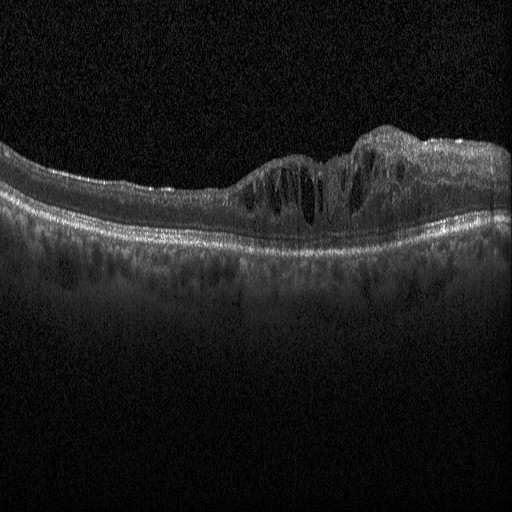
Diagnosis: diabetic macular edema (DME).